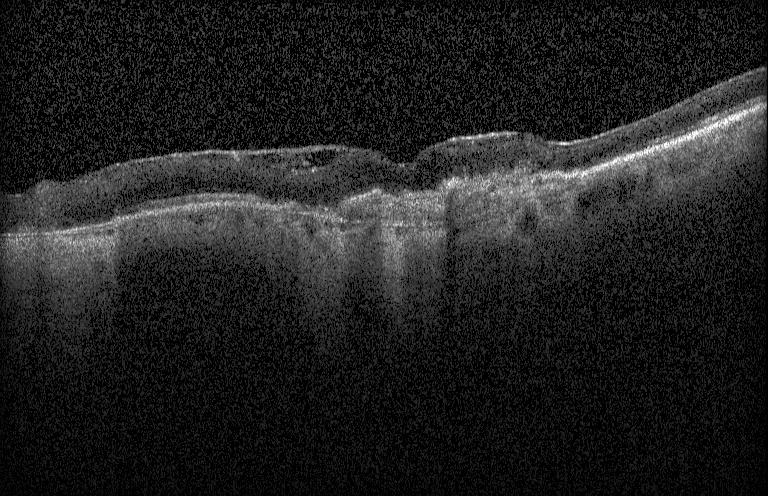
OCT B-scan showing a choroidal neovascular membrane.